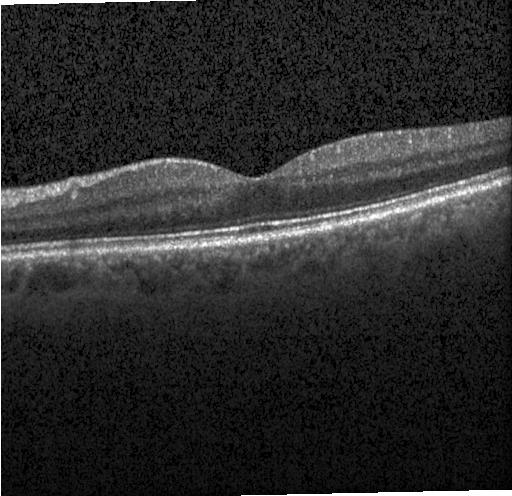
Spectral-domain optical coherence tomography; OCT B-scan; Heidelberg Spectralis
This B-scan demonstrates neither choroidal neovascularization, diabetic macular edema, nor drusen.